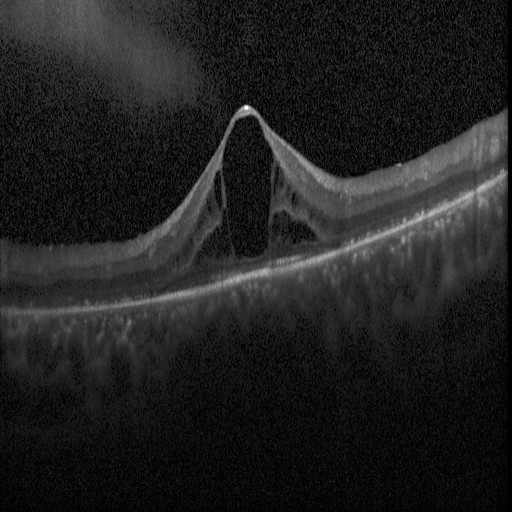 Spectral-domain OCT; macular scan; retinal OCT B-scan; instrument: Heidelberg Spectralis.
Diabetic macular edema (DME).